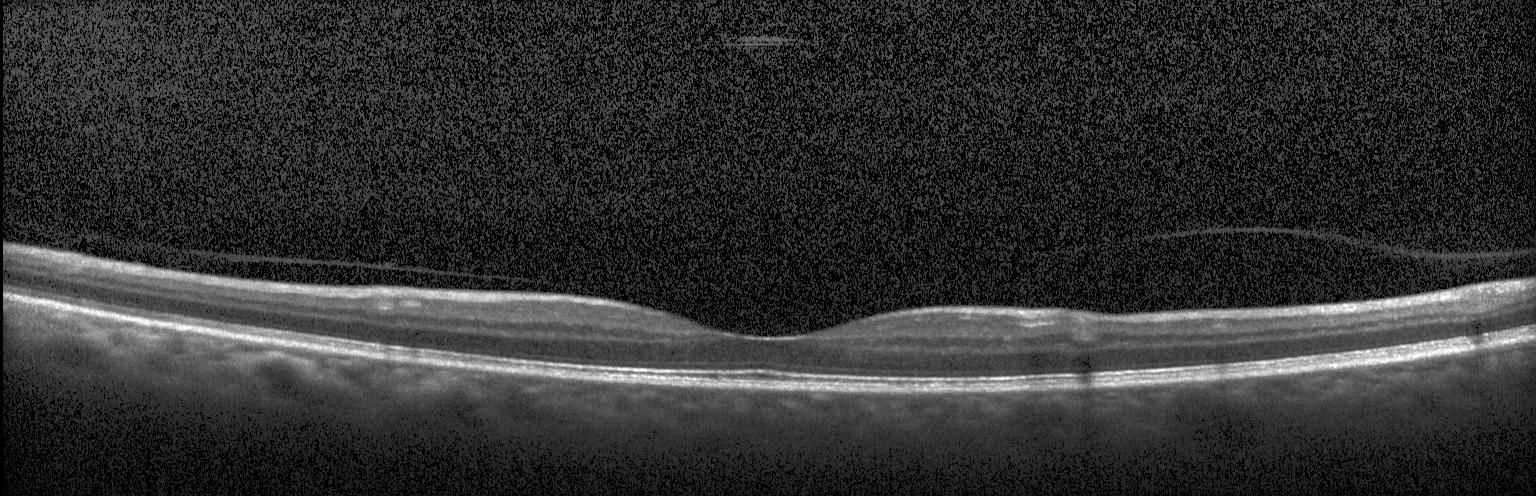
Diagnosis: no choroidal neovascularization, diabetic macular edema, or drusen.